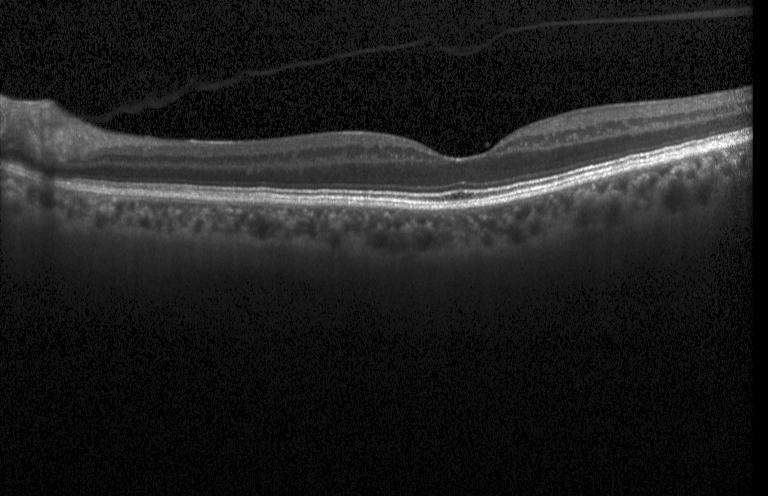 Retinal OCT B-scan — Diagnosis: neither CNV, DME, nor drusen.